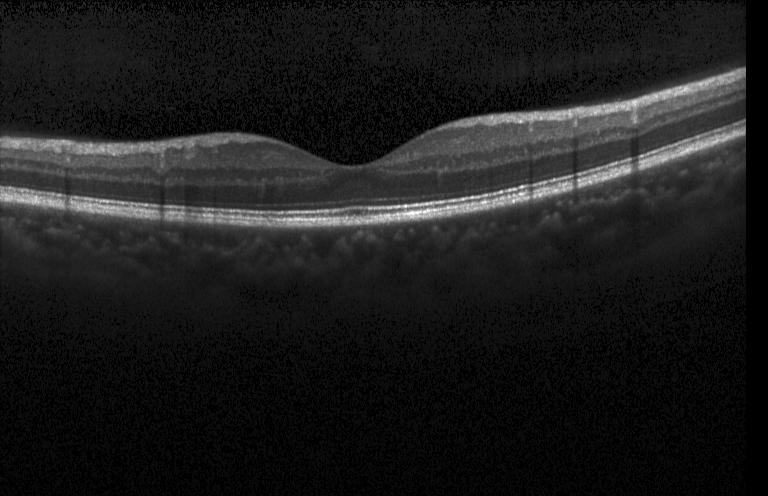
Through the macula · SD-OCT · OCT B-scan
Dx: no choroidal neovascularization, diabetic macular edema, or drusen.